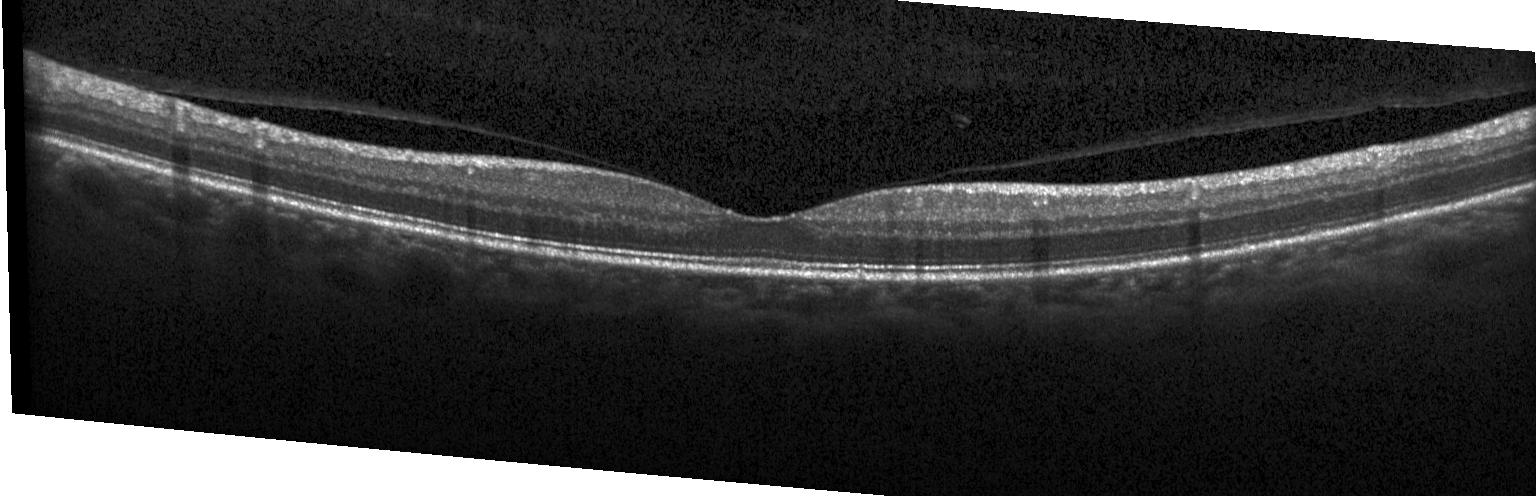 Spectral-domain optical coherence tomography · Heidelberg Spectralis OCT system · OCT line scan.
Impression: no evidence of choroidal neovascularization, diabetic macular edema, or drusen.